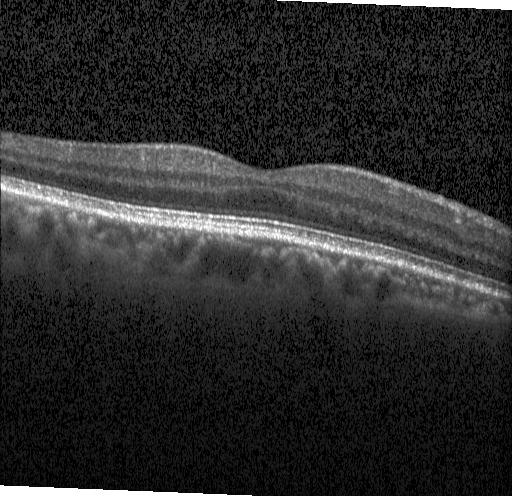
Retinal OCT cross-section · fovea-centered — Finding: no choroidal neovascularization, diabetic macular edema, or drusen.